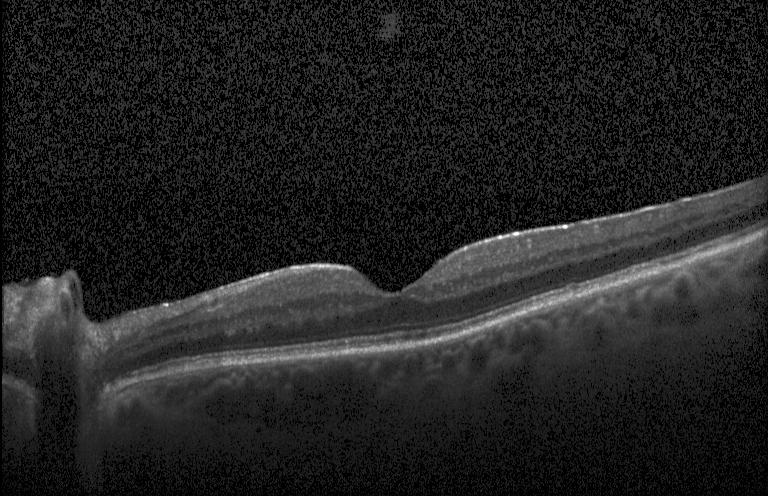
Dx: no CNV, DME, or drusen.